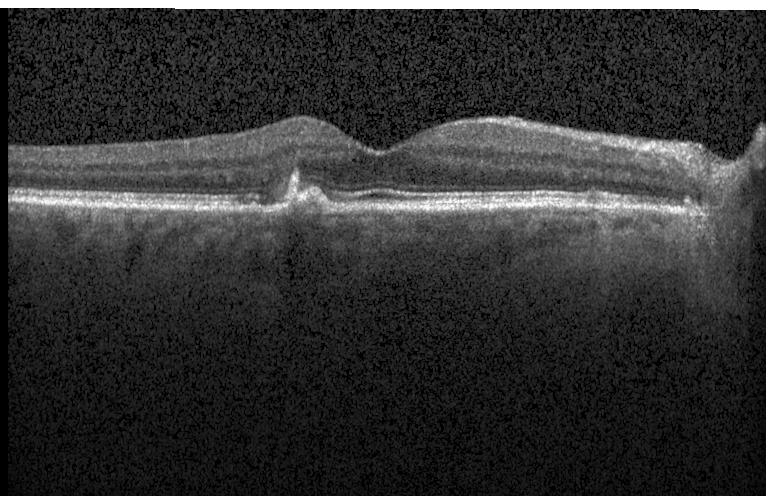 Instrument: Heidelberg Spectralis. Retinal OCT cross-section. Spectral-domain optical coherence tomography
Finding: a choroidal neovascular membrane.